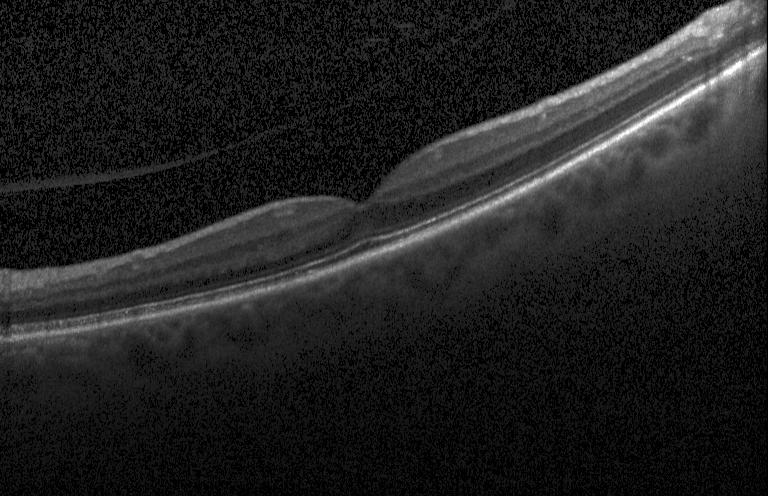

Finding: no choroidal neovascularization, diabetic macular edema, or drusen.